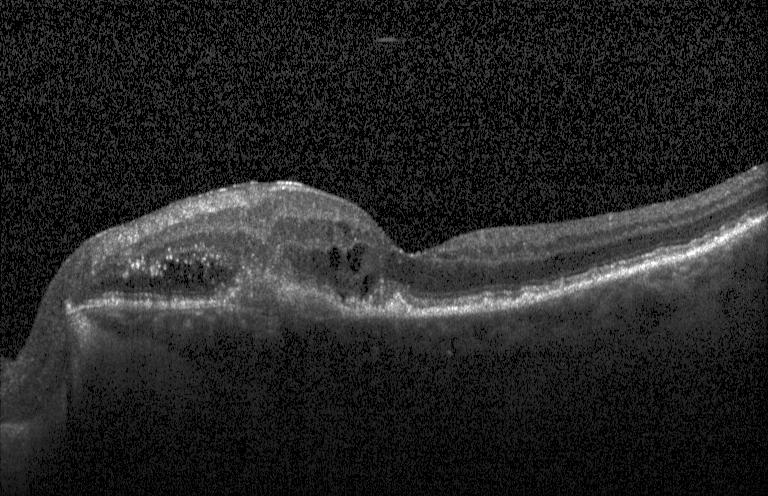

Impression: choroidal neovascularization (CNV).